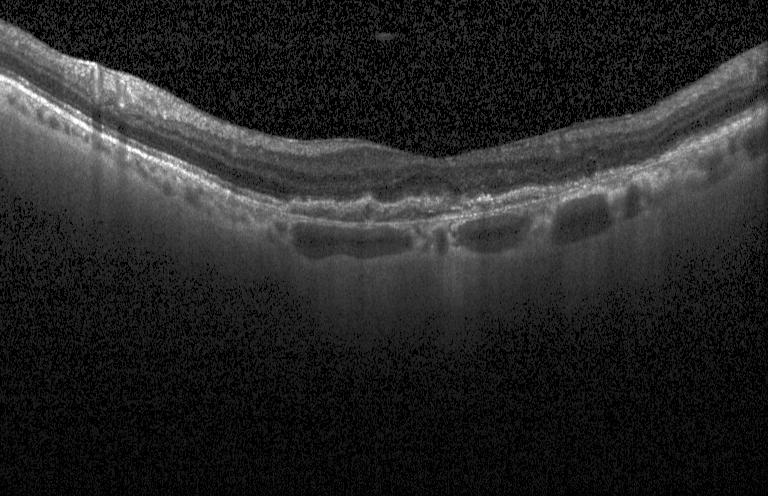

Acquired on a Heidelberg Spectralis. Optical coherence tomography B-scan. Spectral-domain optical coherence tomography — Finding: CNV.